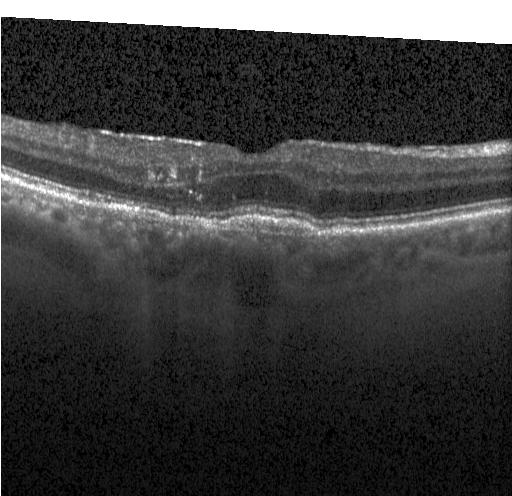
OCT finding: a choroidal neovascular membrane.